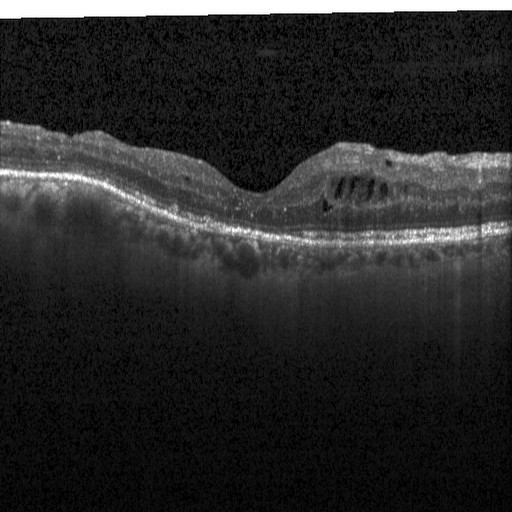

Retinal OCT cross-section
Finding: diabetic macular edema (DME).